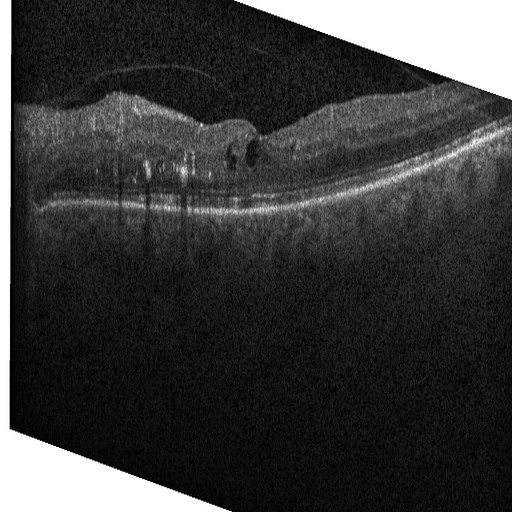 SD-OCT · optical coherence tomography B-scan · Heidelberg Spectralis OCT system · horizontal scan through the fovea.
Finding: diabetic macular edema.